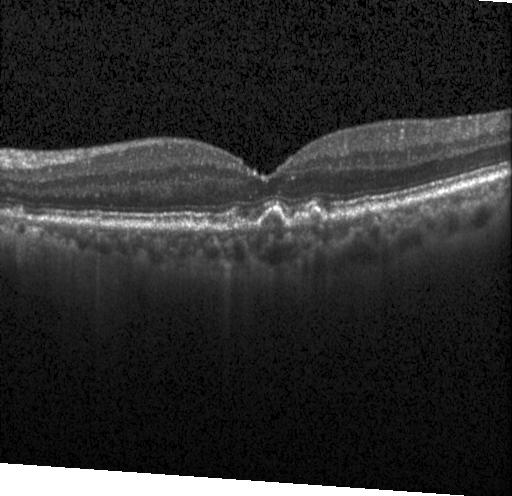

Impression: multiple drusen.